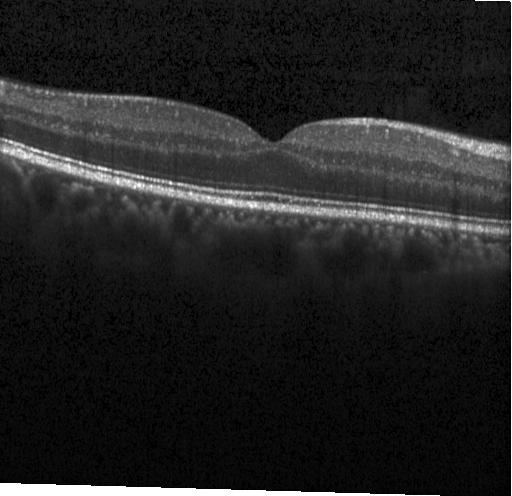 Retinal OCT B-scan. SD-OCT. Horizontal scan through the fovea. The scan shows no evidence of choroidal neovascularization, diabetic macular edema, or drusen.